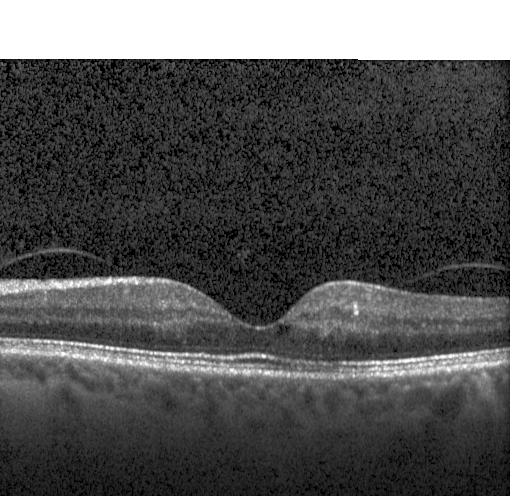
Instrument: Heidelberg Spectralis, optical coherence tomography B-scan
Impression: diabetic macular edema (DME).